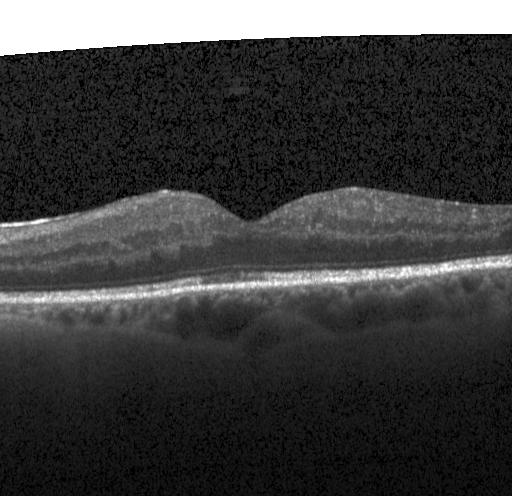

Finding: no choroidal neovascularization, no diabetic macular edema, and no drusen.